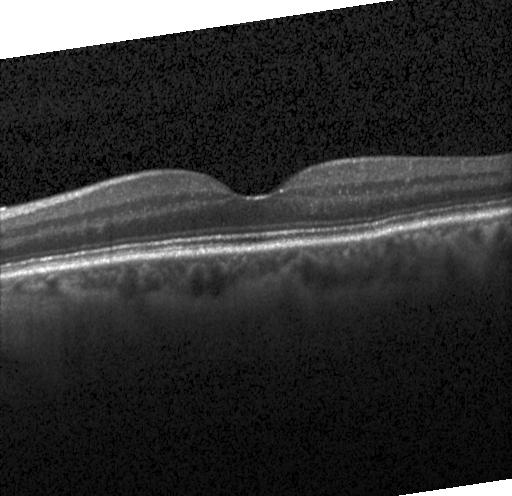

Dx: neither choroidal neovascularization, diabetic macular edema, nor drusen.